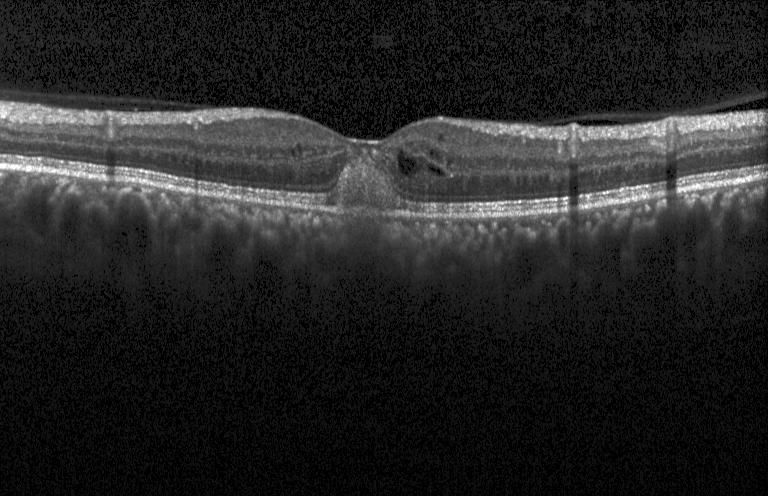 Through the macula, acquired on a Heidelberg Spectralis, retinal OCT B-scan, spectral-domain OCT
Choroidal neovascularization.